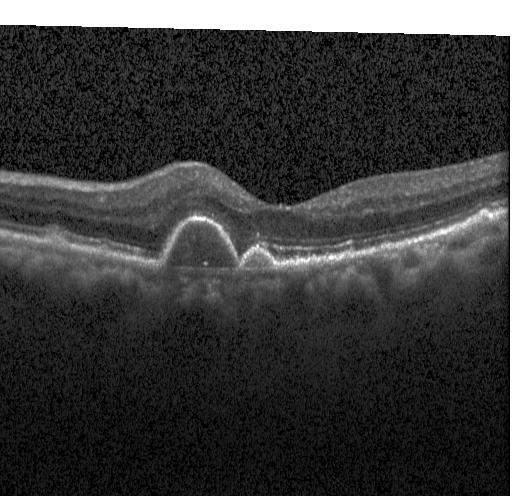

OCT line scan · spectral-domain OCT · Heidelberg Spectralis OCT system. The scan shows multiple drusen.